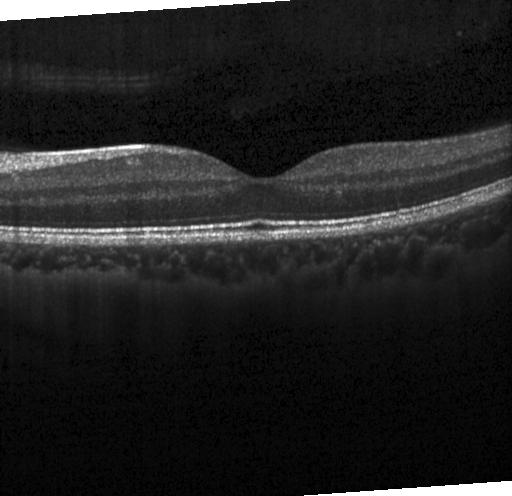 OCT B-scan. Instrument: Heidelberg Spectralis. Through the macula.
Neither choroidal neovascularization, diabetic macular edema, nor drusen.